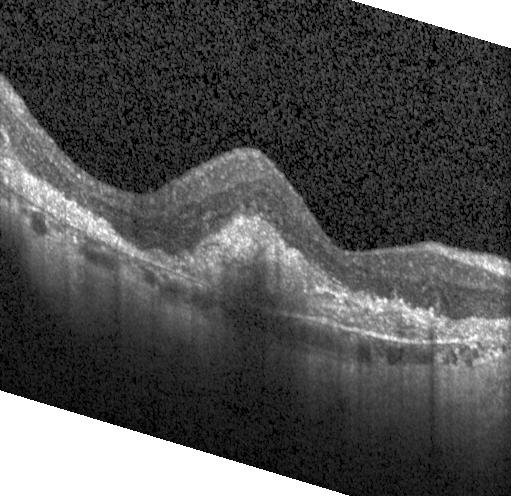
Optical coherence tomography B-scan; instrument: Heidelberg Spectralis. Finding: a choroidal neovascular membrane.